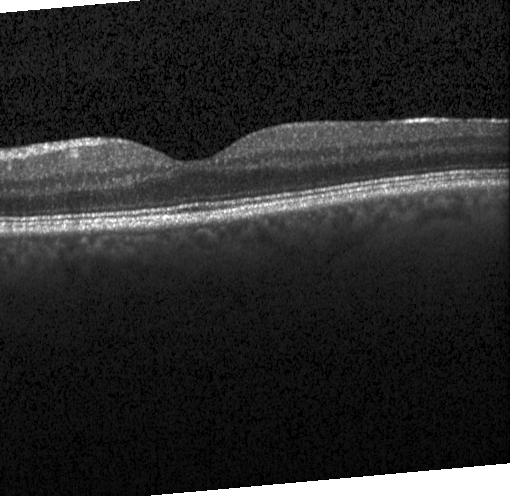

The scan shows no choroidal neovascularization, no diabetic macular edema, and no drusen.